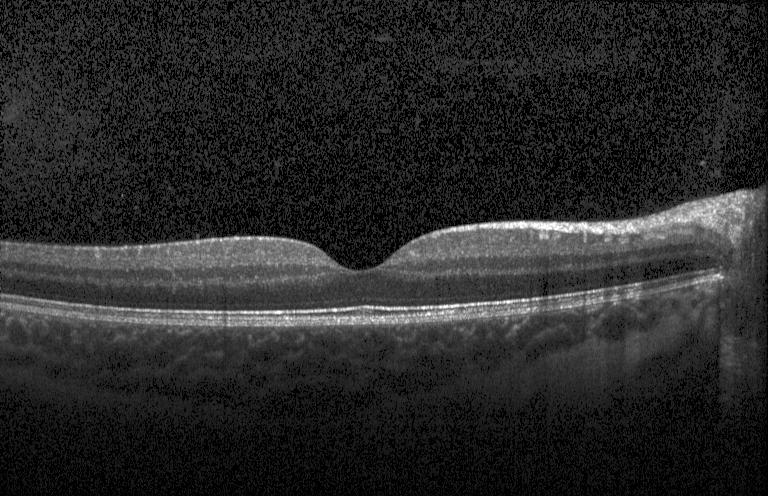

Optical coherence tomography scan, horizontal scan through the fovea, spectral-domain OCT, Heidelberg Spectralis — OCT finding: no CNV, DME, or drusen.